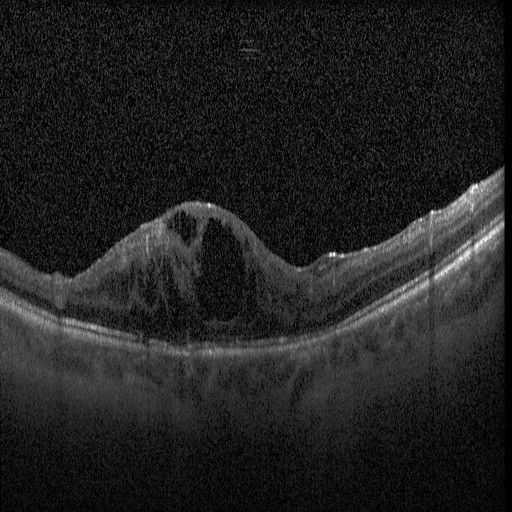

OCT finding: diabetic macular edema.